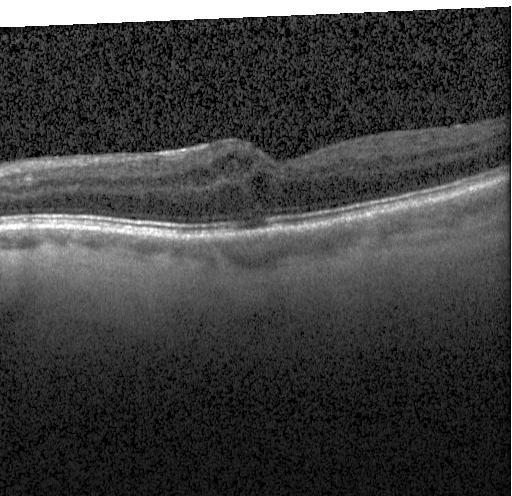 OCT B-scan · SD-OCT
The scan shows diabetic macular edema (DME).